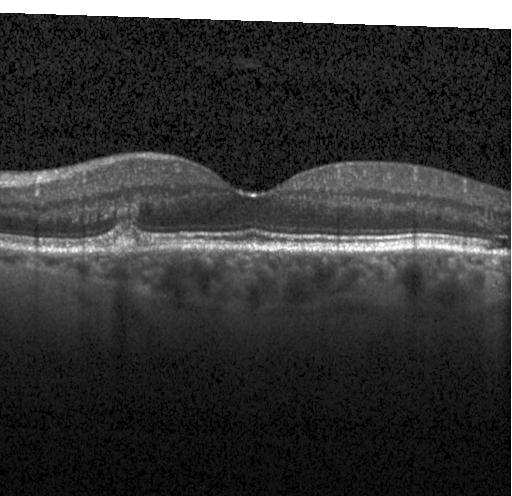 Heidelberg Spectralis; retinal OCT B-scan; centered on the fovea — Finding: sub-RPE drusenoid deposits.